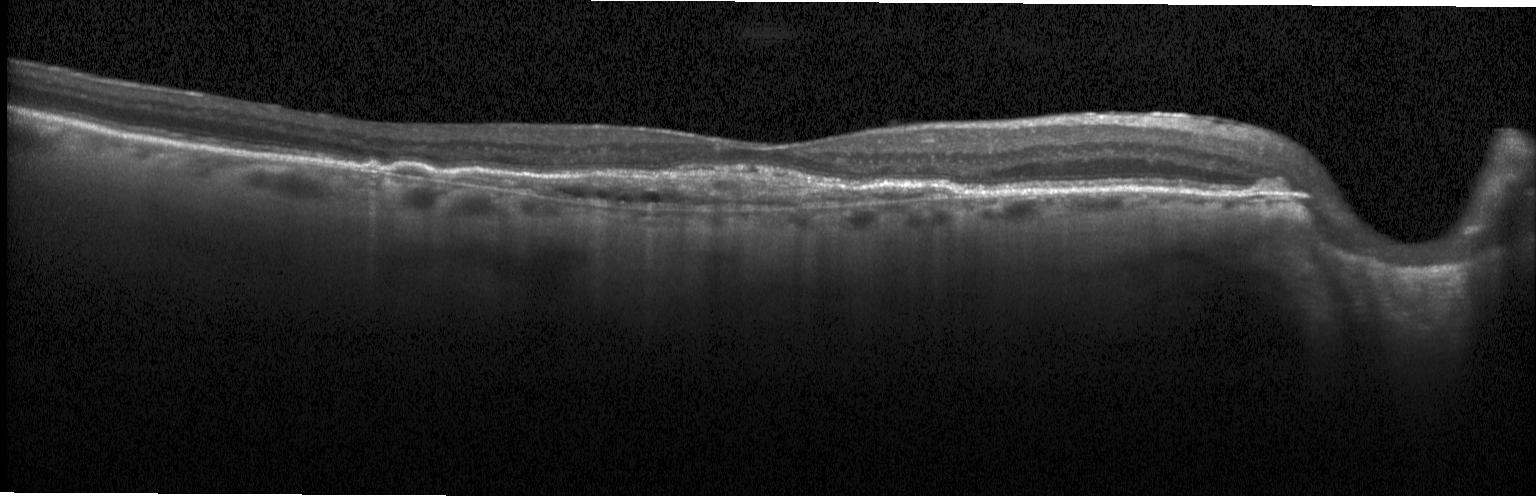

Through the macula; OCT B-scan; SD-OCT; Heidelberg Spectralis OCT system — Diagnosis: CNV.